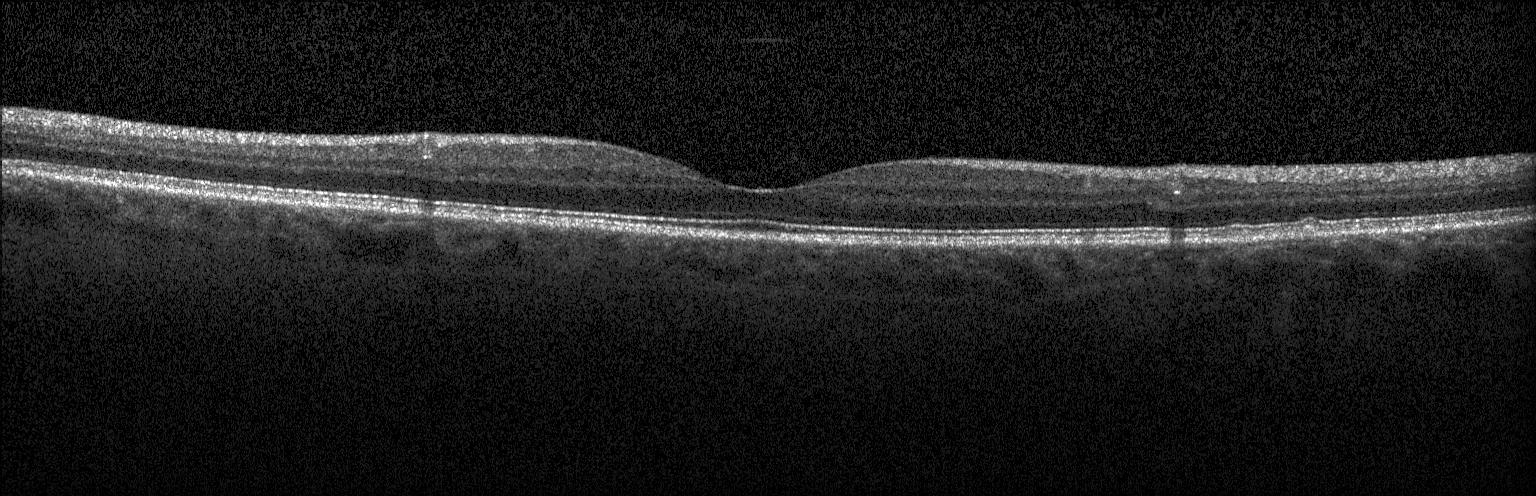 Retinal OCT B-scan
Dx: neither choroidal neovascularization, diabetic macular edema, nor drusen.